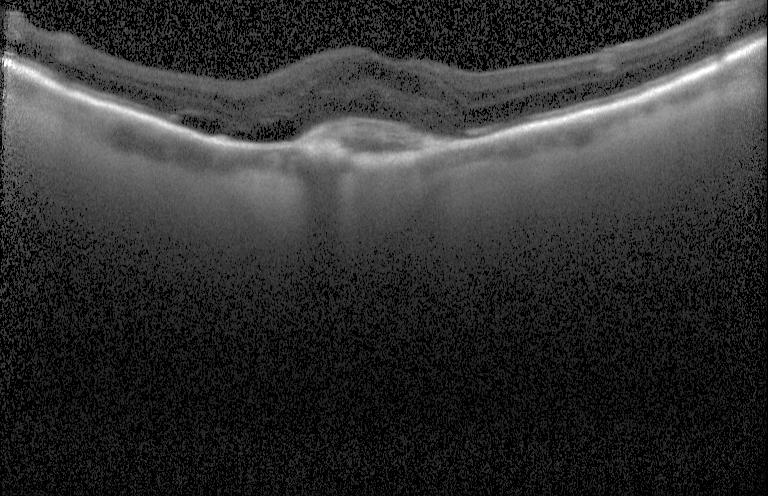

This B-scan demonstrates choroidal neovascularization (CNV).